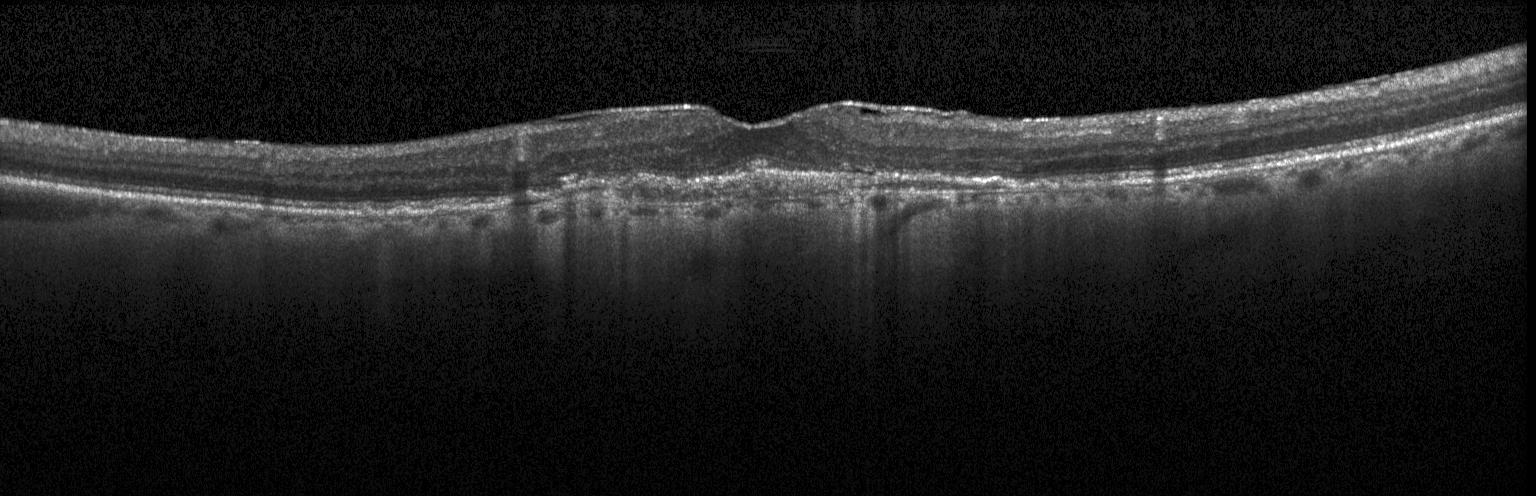 Centered on the fovea. Spectral-domain OCT. Heidelberg Spectralis. Retinal OCT cross-section — Finding: choroidal neovascularization (CNV).